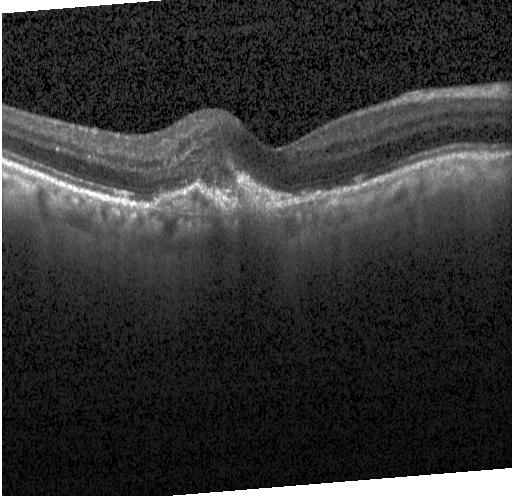 Fovea-centered; optical coherence tomography B-scan. Dx: a choroidal neovascular membrane.